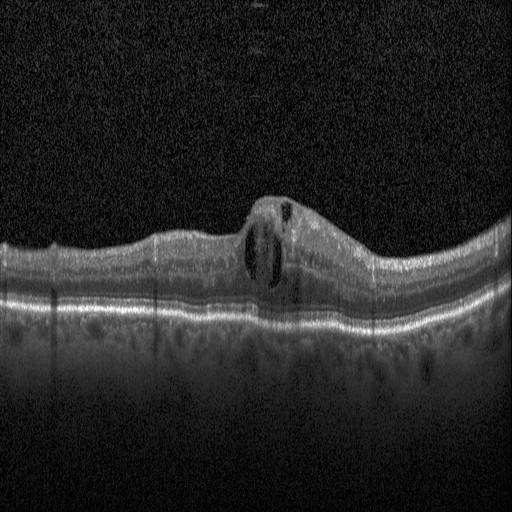
Spectral-domain OCT, OCT line scan, Heidelberg Spectralis OCT system, horizontal scan through the fovea — Finding: DME.